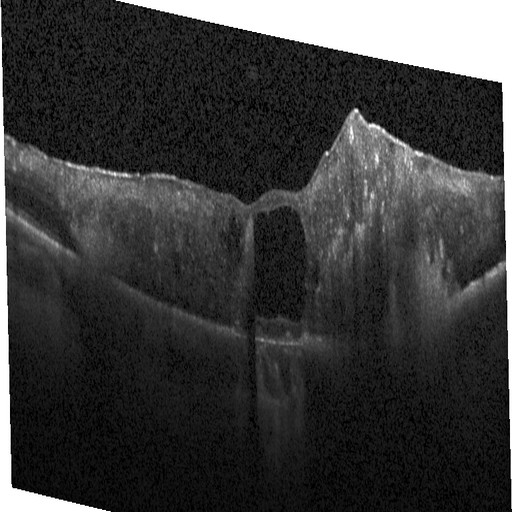 OCT scan showing DME.